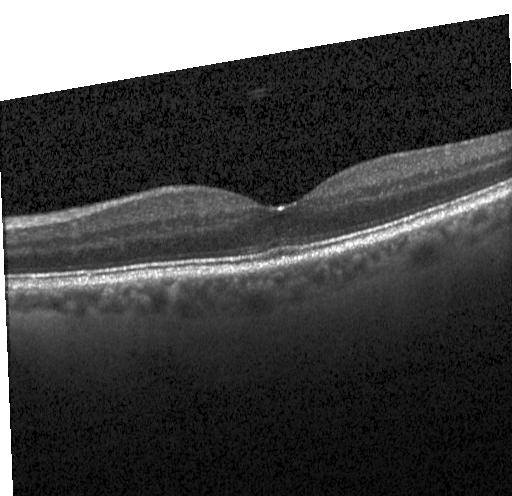
Optical coherence tomography B-scan.
Impression: no CNV, no DME, and no drusen.